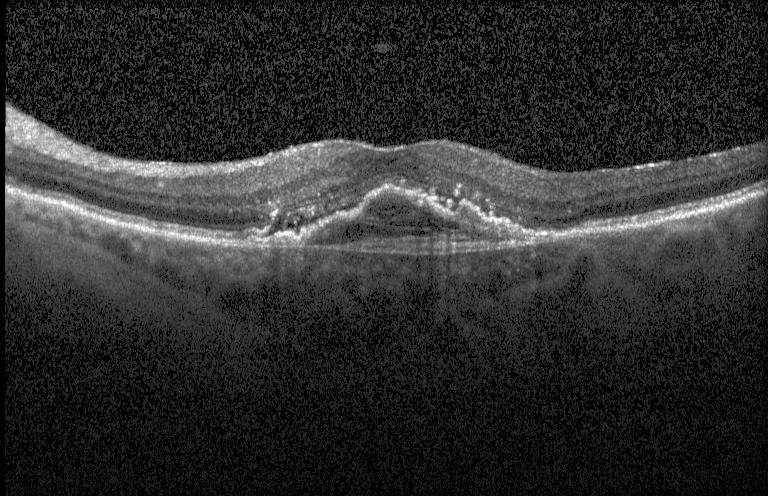
A choroidal neovascular membrane.